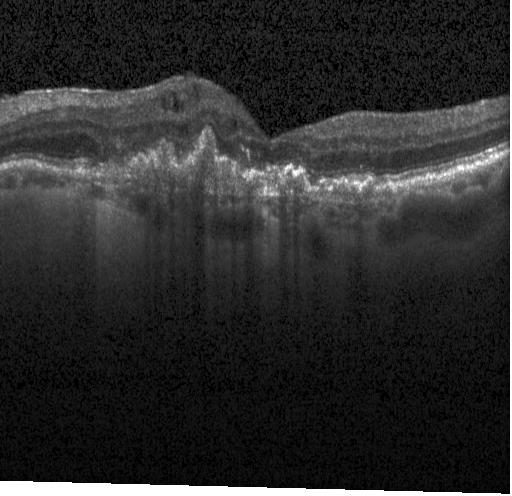
Dx: CNV.